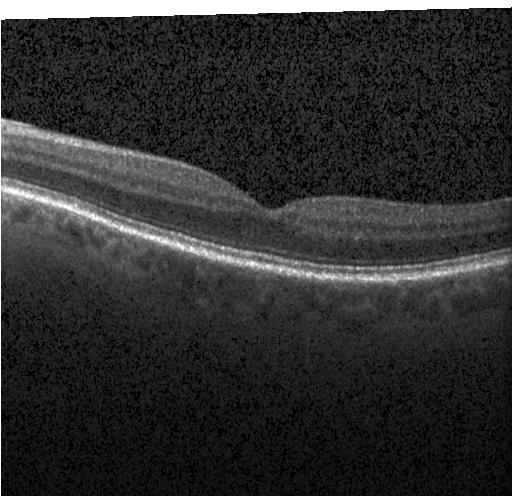 Optical coherence tomography scan — Dx: no evidence of choroidal neovascularization, diabetic macular edema, or drusen.